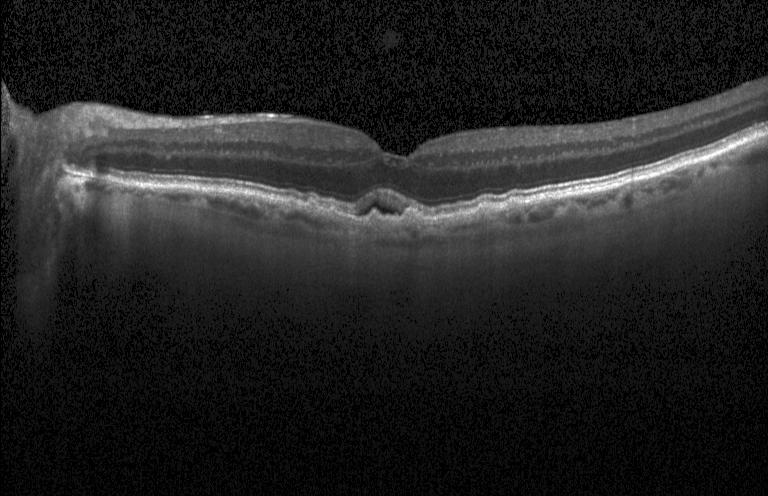

Impression: choroidal neovascularization.